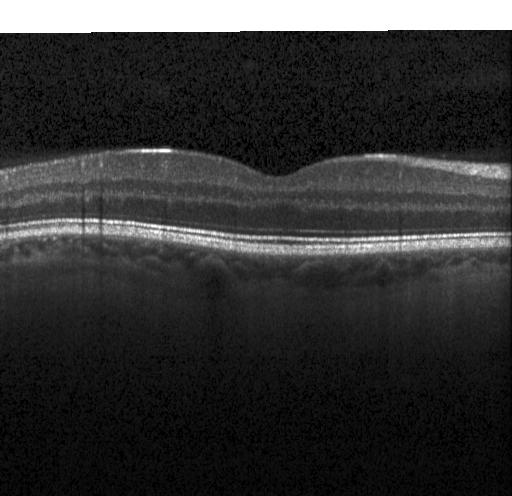

Spectral-domain optical coherence tomography; acquired on a Heidelberg Spectralis; OCT B-scan; horizontal scan through the fovea
OCT finding: neither choroidal neovascularization, diabetic macular edema, nor drusen.